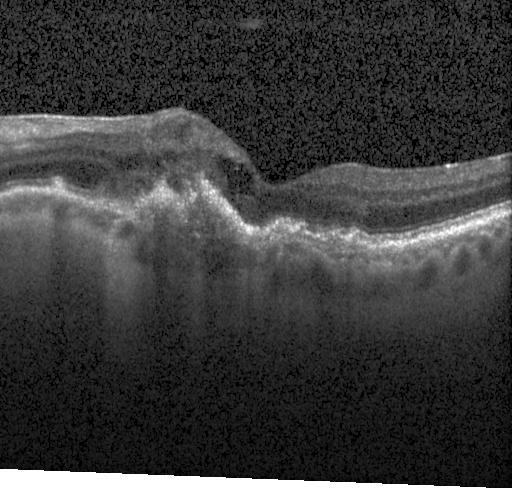 Retinal OCT B-scan · Heidelberg Spectralis.
Impression: choroidal neovascularization (CNV).